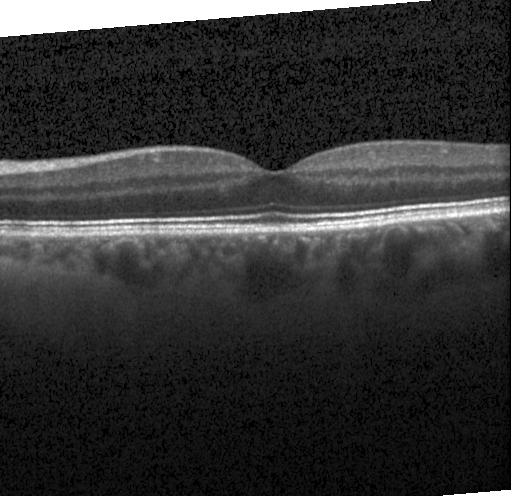
Impression: neither choroidal neovascularization, diabetic macular edema, nor drusen.